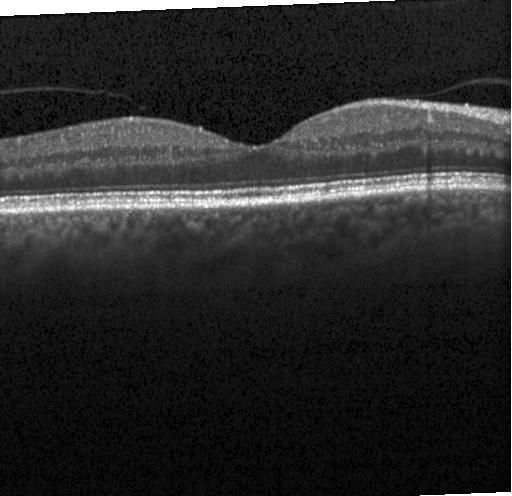
Macular OCT: no evidence of CNV, DME, or drusen.